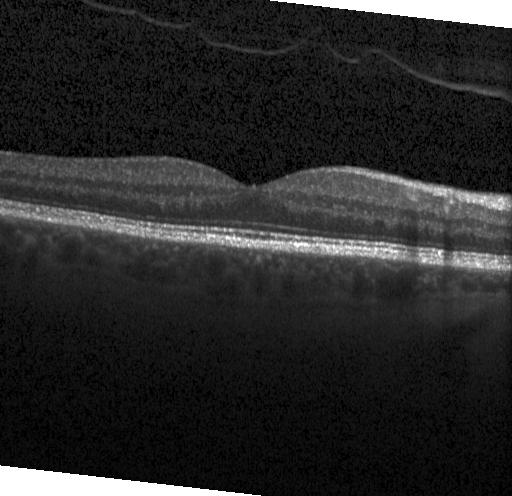
Centered on the fovea. Heidelberg Spectralis OCT system. OCT B-scan. Spectral-domain OCT
Finding: no evidence of choroidal neovascularization, diabetic macular edema, or drusen.